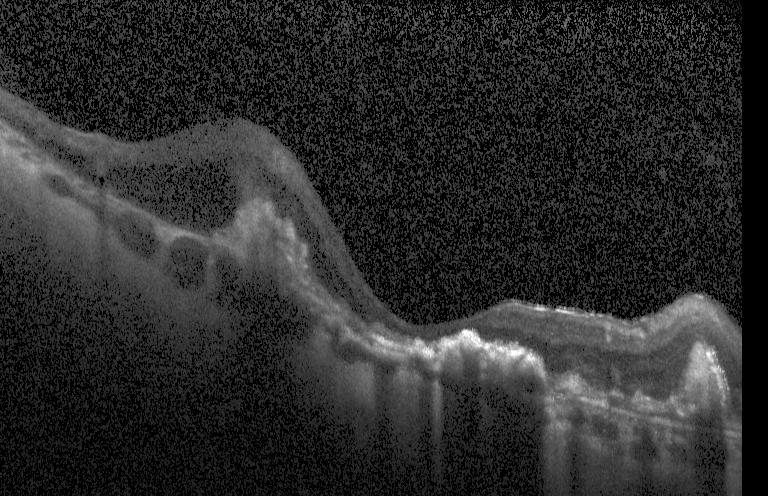 SD-OCT · OCT line scan. Diagnosis: a choroidal neovascular membrane.